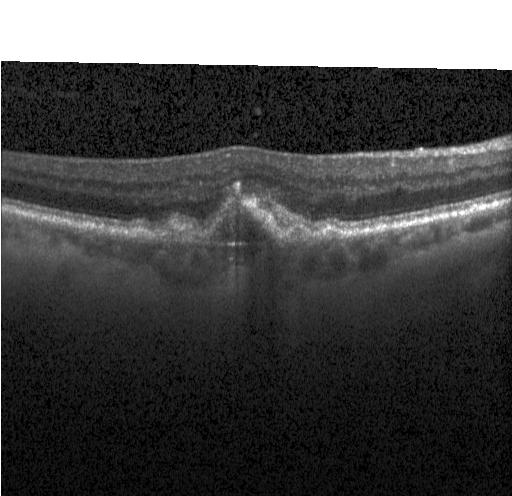
Optical coherence tomography B-scan.
Macular OCT: a choroidal neovascular membrane.